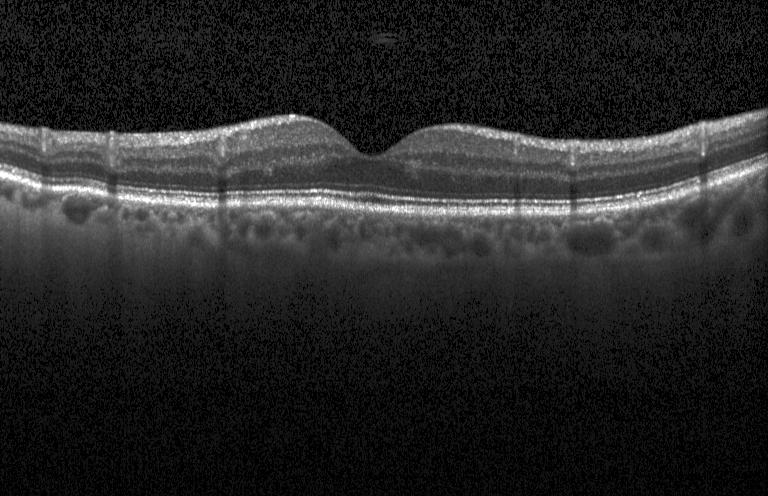
SD-OCT · optical coherence tomography scan · horizontal scan through the fovea · instrument: Heidelberg Spectralis. Impression: neither choroidal neovascularization, diabetic macular edema, nor drusen.